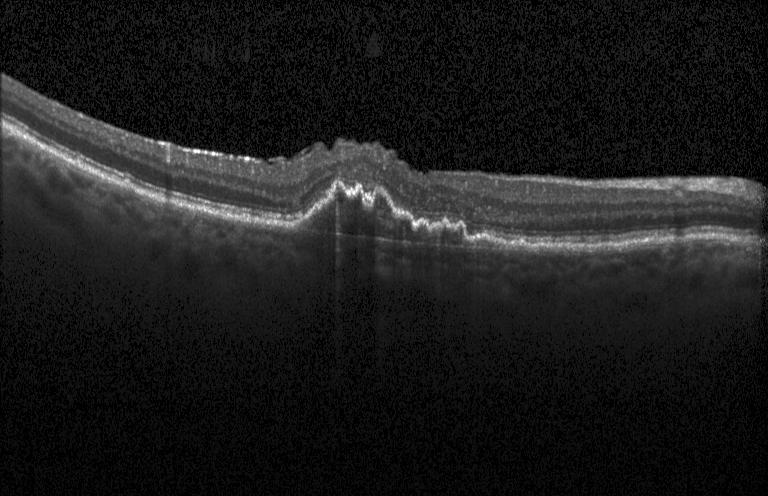

Retinal OCT cross-section. Horizontal scan through the fovea. Heidelberg Spectralis OCT system.
Diagnosis: choroidal neovascularization (CNV).